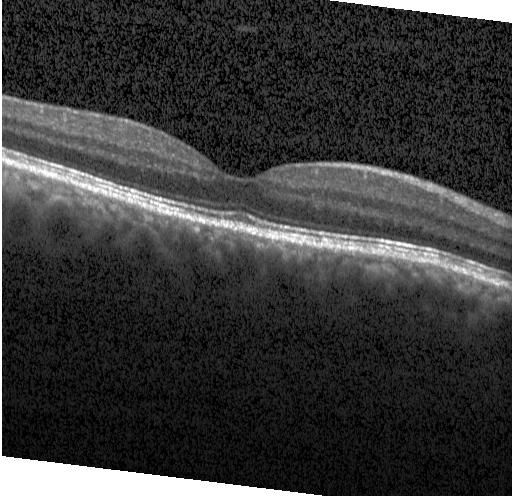
Spectral-domain optical coherence tomography. Retinal OCT cross-section. Instrument: Heidelberg Spectralis. OCT finding: no CNV, no DME, and no drusen.